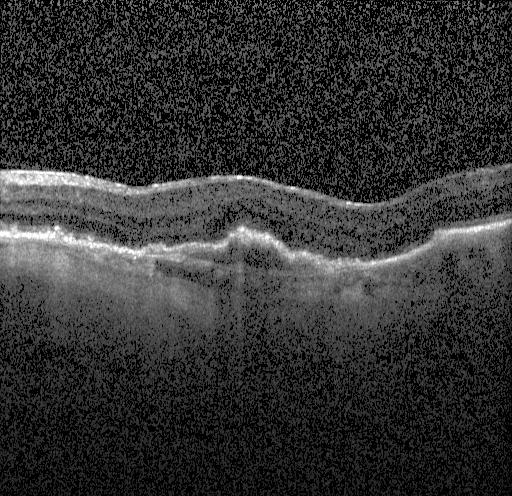

The scan shows choroidal neovascularization (CNV).